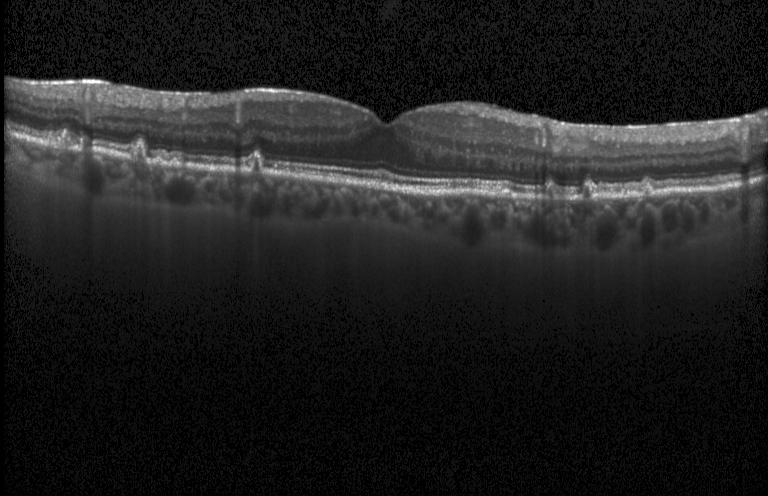

Optical coherence tomography B-scan · macular scan · spectral-domain OCT · Heidelberg Spectralis OCT system.
This B-scan demonstrates sub-RPE drusenoid deposits.